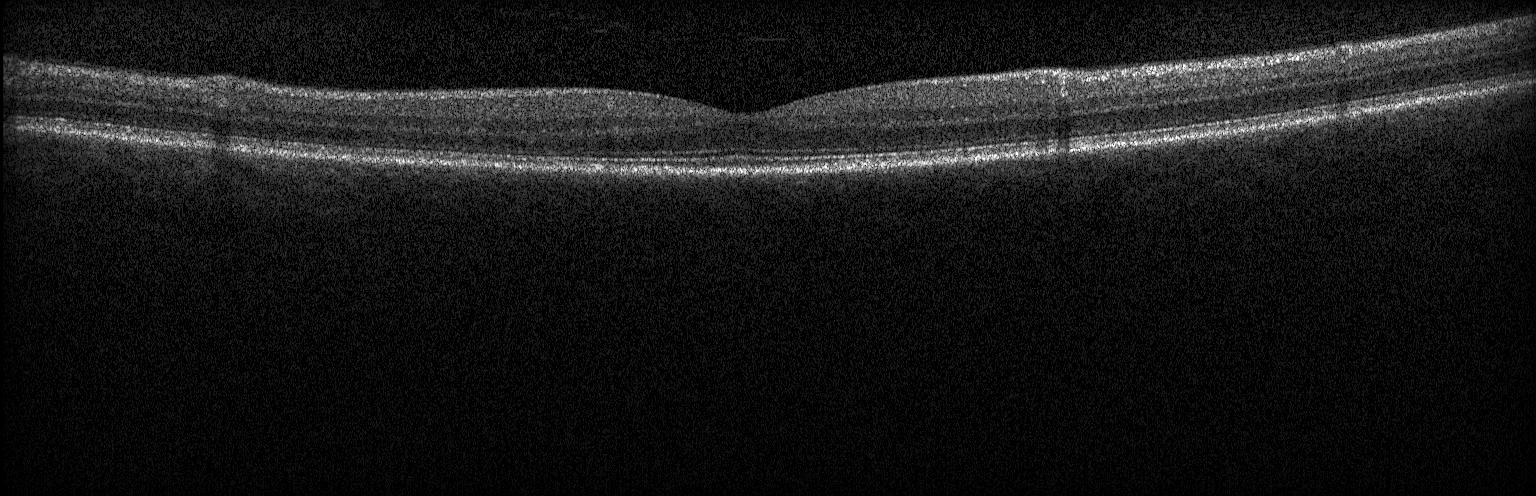 Acquired on a Heidelberg Spectralis; spectral-domain optical coherence tomography; macular scan; optical coherence tomography scan.
This B-scan demonstrates no CNV, no DME, and no drusen.